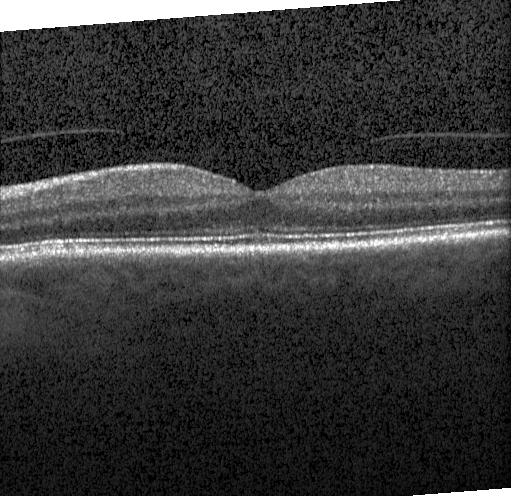
OCT B-scan showing no CNV, DME, or drusen.